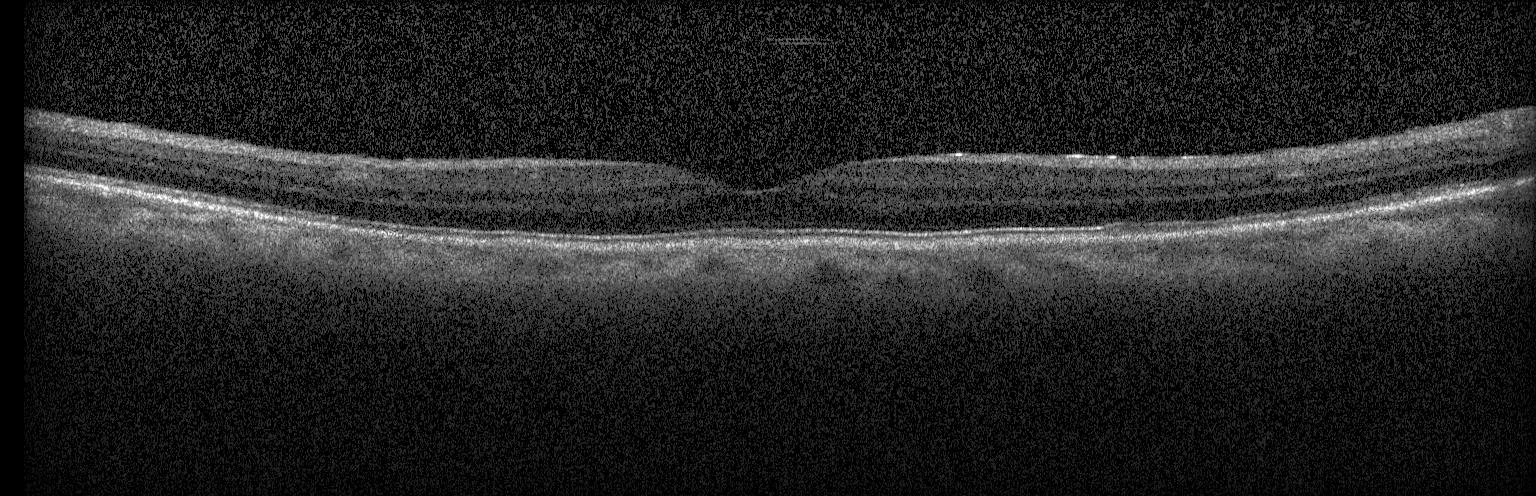

Through the macula. Optical coherence tomography B-scan. Acquired on a Heidelberg Spectralis
This B-scan demonstrates neither choroidal neovascularization, diabetic macular edema, nor drusen.